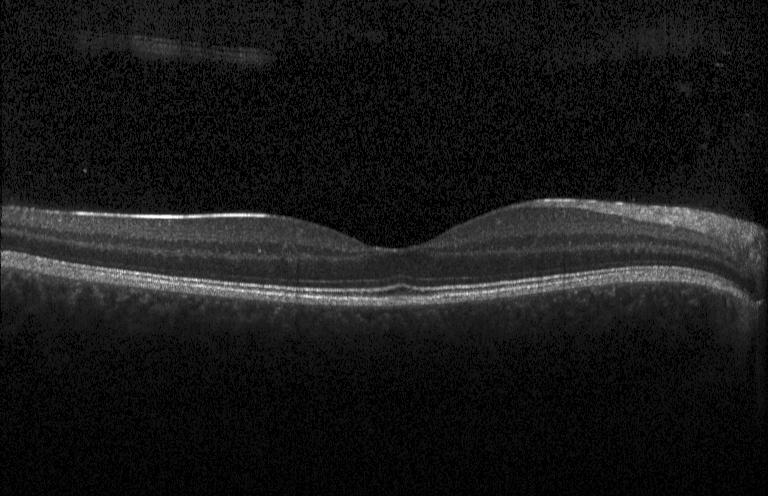

Macular scan. Heidelberg Spectralis. OCT line scan.
The scan shows no CNV, no DME, and no drusen.